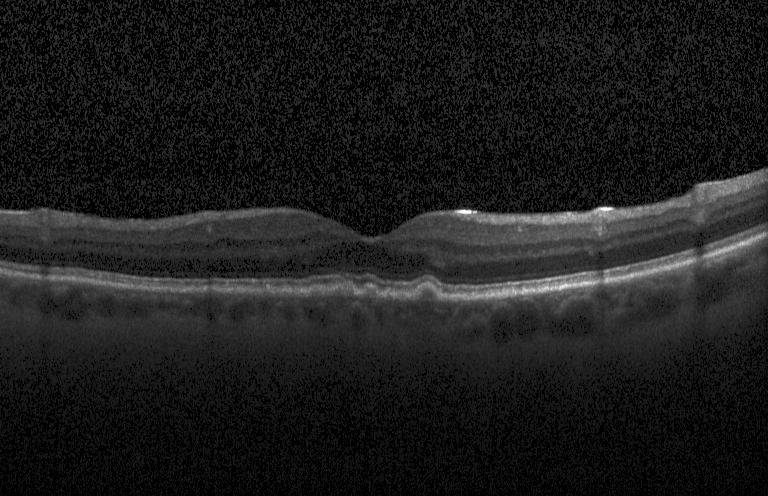 SD-OCT. OCT B-scan — Impression: drusen.